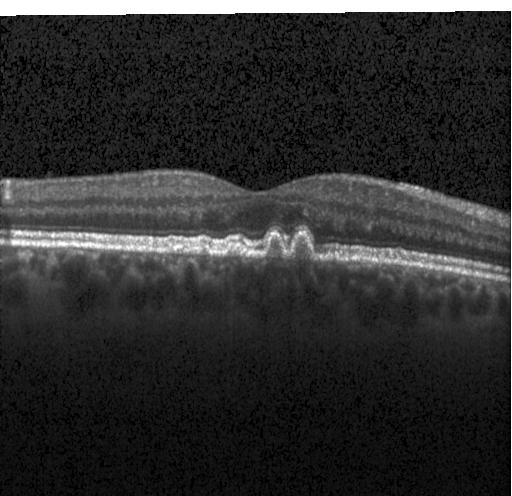

Macular scan. Instrument: Heidelberg Spectralis. Retinal OCT cross-section — OCT finding: drusen.